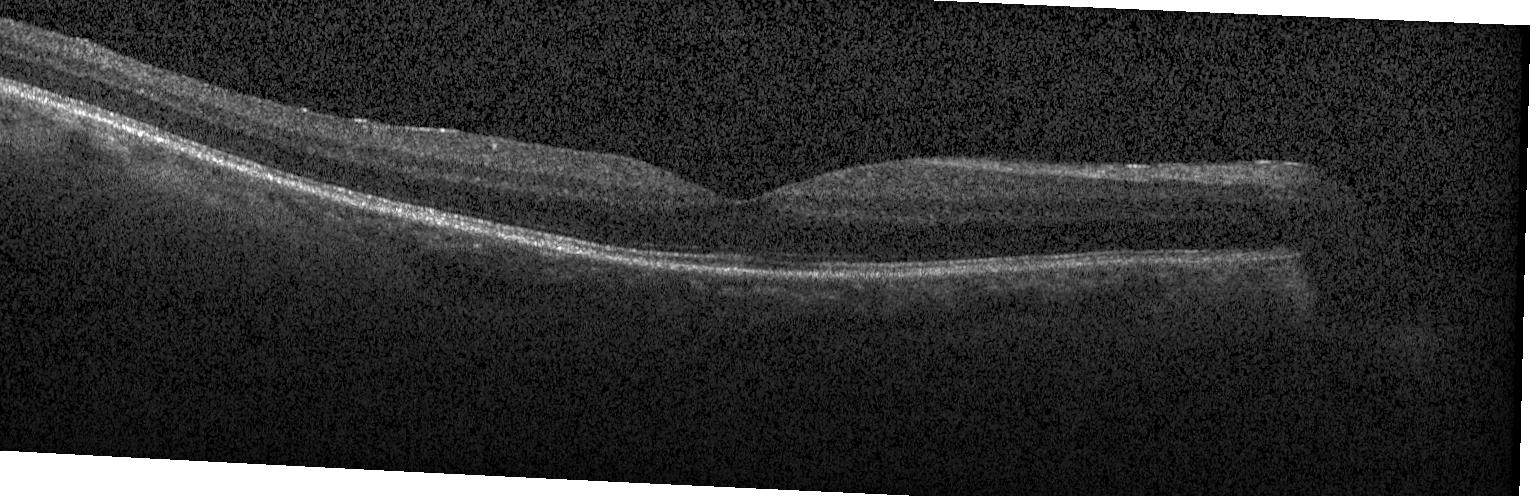
OCT B-scan — The scan shows no choroidal neovascularization, no diabetic macular edema, and no drusen.